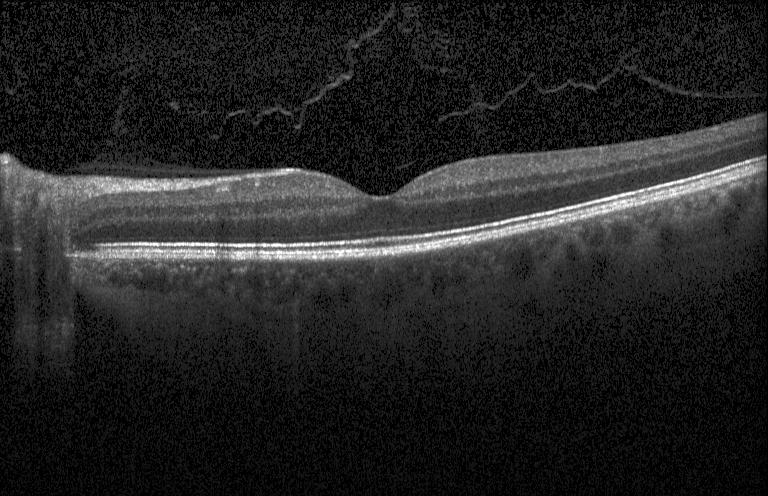
Optical coherence tomography scan · fovea-centered · SD-OCT — Impression: no evidence of choroidal neovascularization, diabetic macular edema, or drusen.